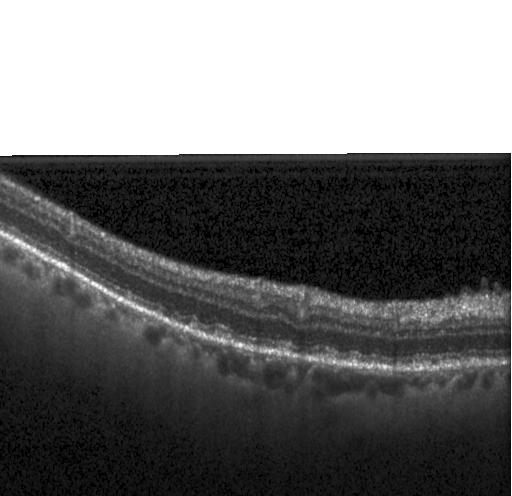 OCT B-scan, fovea-centered, SD-OCT
Impression: multiple drusen.